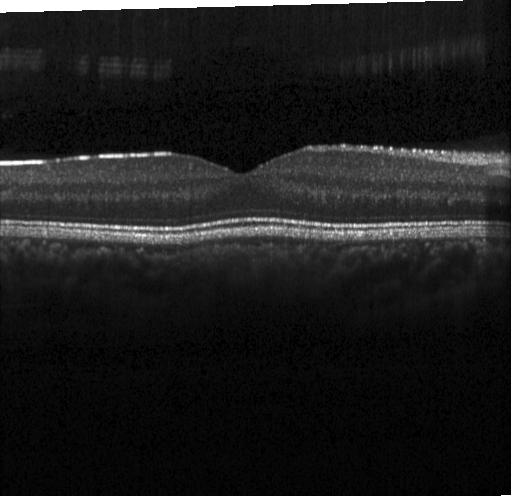
Macular scan, acquired on a Heidelberg Spectralis, OCT B-scan — The scan shows neither CNV, DME, nor drusen.